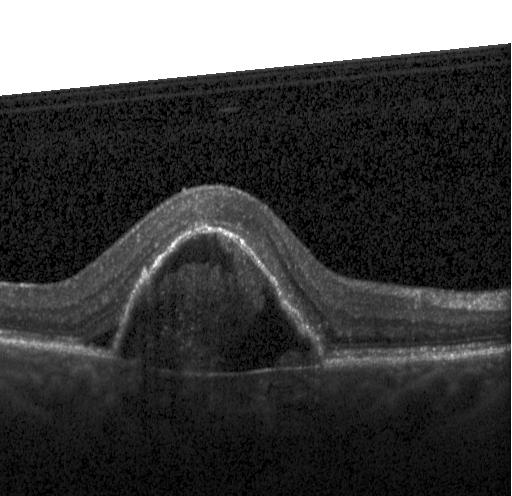 OCT line scan, fovea-centered.
Diagnosis: a choroidal neovascular membrane.